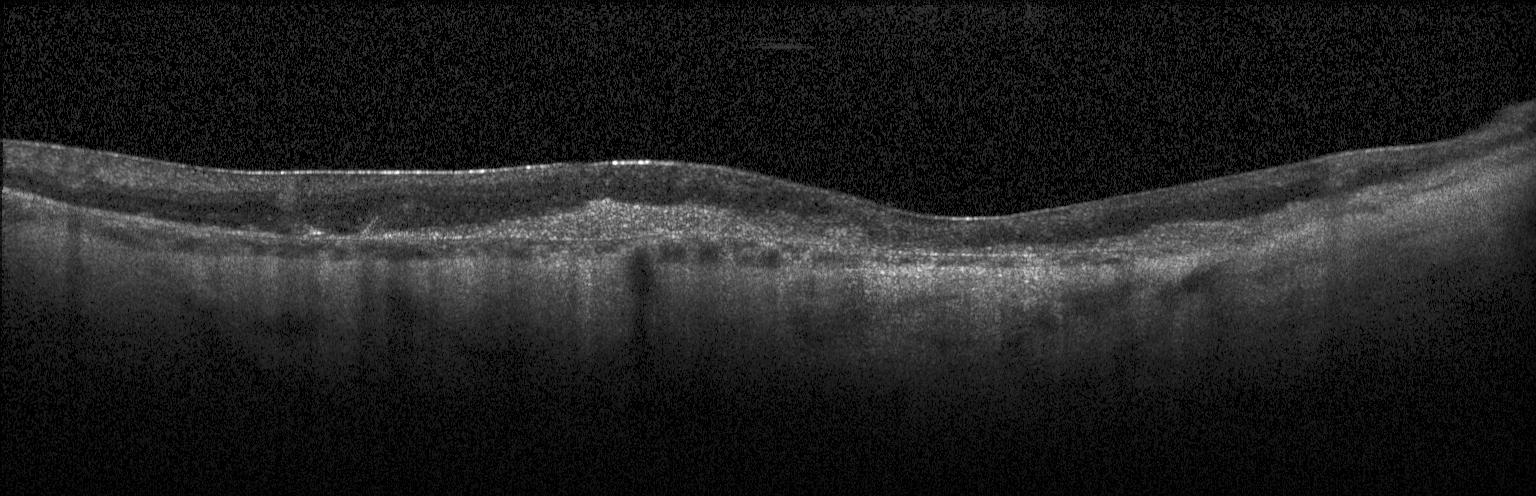
Spectral-domain OCT, fovea-centered, Heidelberg Spectralis, retinal OCT cross-section
Macular OCT: a choroidal neovascular membrane.